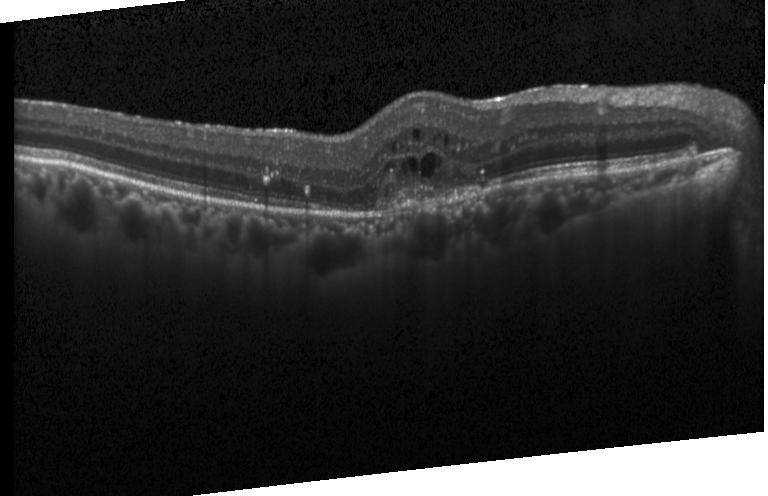

Retinal OCT cross-section — This B-scan demonstrates CNV.